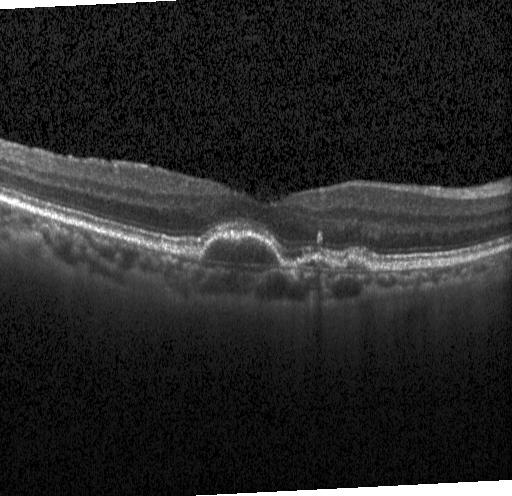 Optical coherence tomography B-scan — A choroidal neovascular membrane.